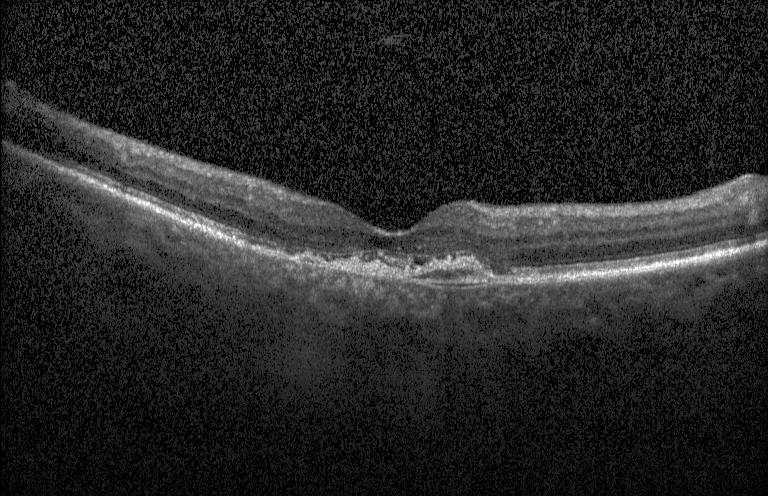 OCT line scan — OCT finding: a choroidal neovascular membrane.